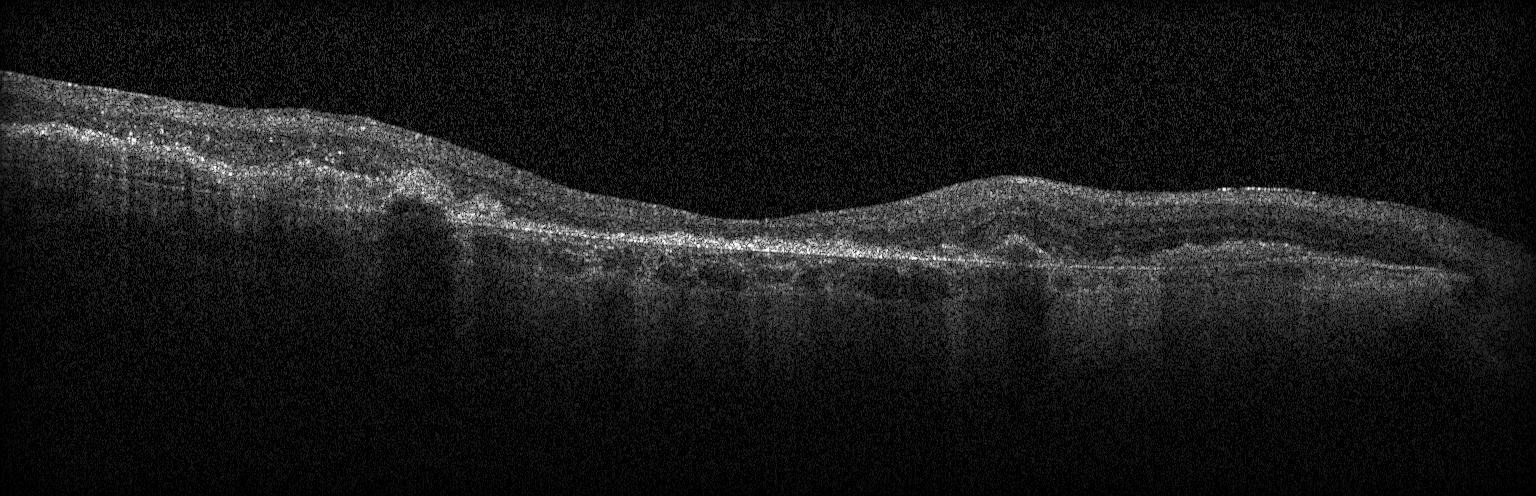

OCT B-scan showing CNV.